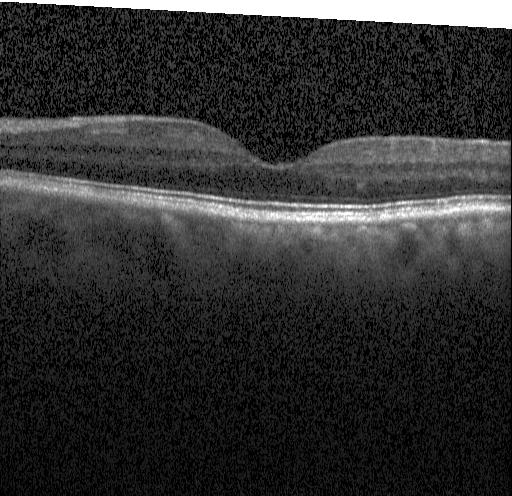
OCT line scan; instrument: Heidelberg Spectralis; horizontal scan through the fovea.
This B-scan demonstrates neither choroidal neovascularization, diabetic macular edema, nor drusen.